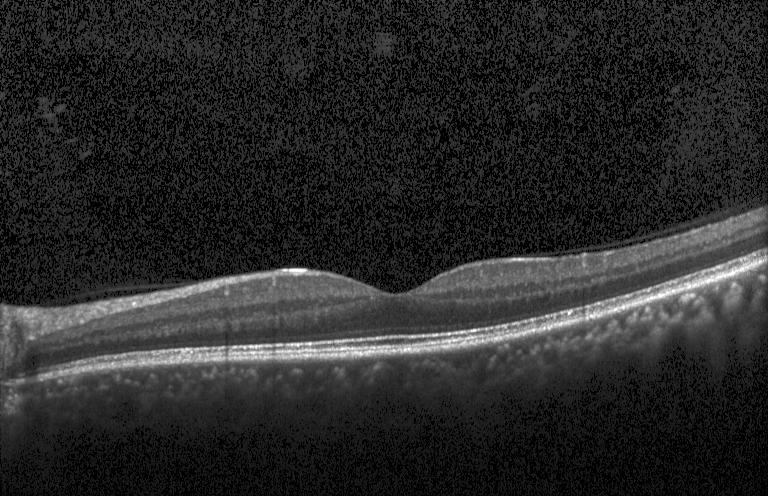
Optical coherence tomography B-scan. Finding: neither CNV, DME, nor drusen.